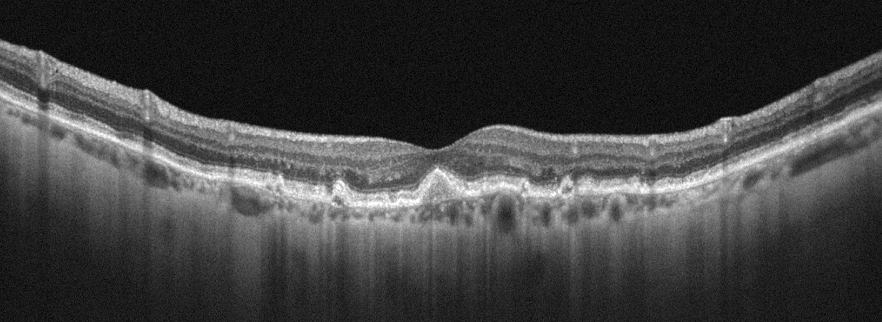

Retinal OCT B-scan · oculus sinister. OCT finding: age-related macular degeneration.